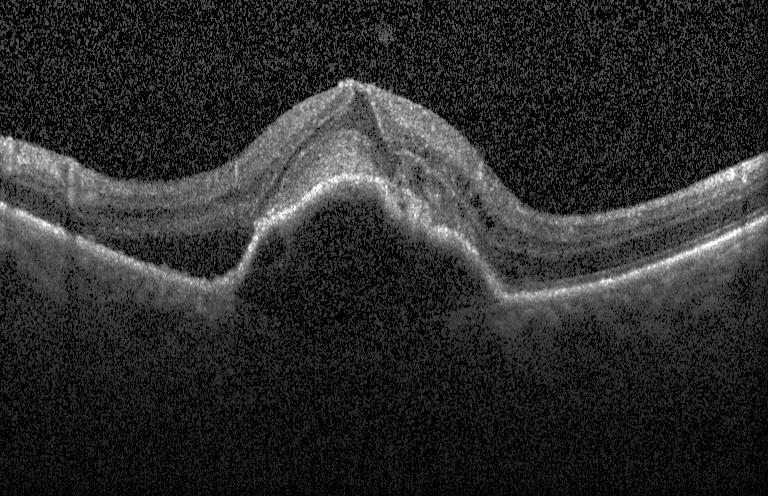
Diagnosis: a choroidal neovascular membrane.